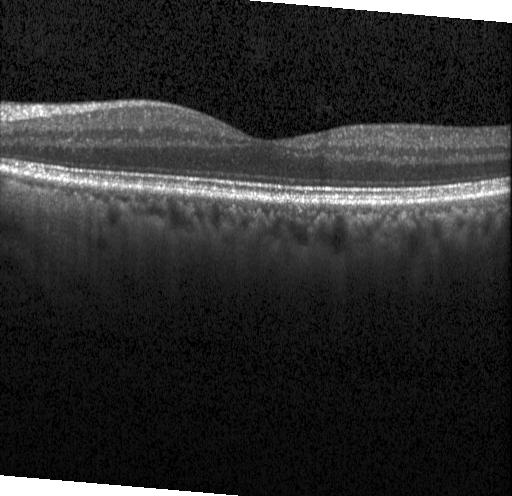
Impression: no CNV, DME, or drusen.